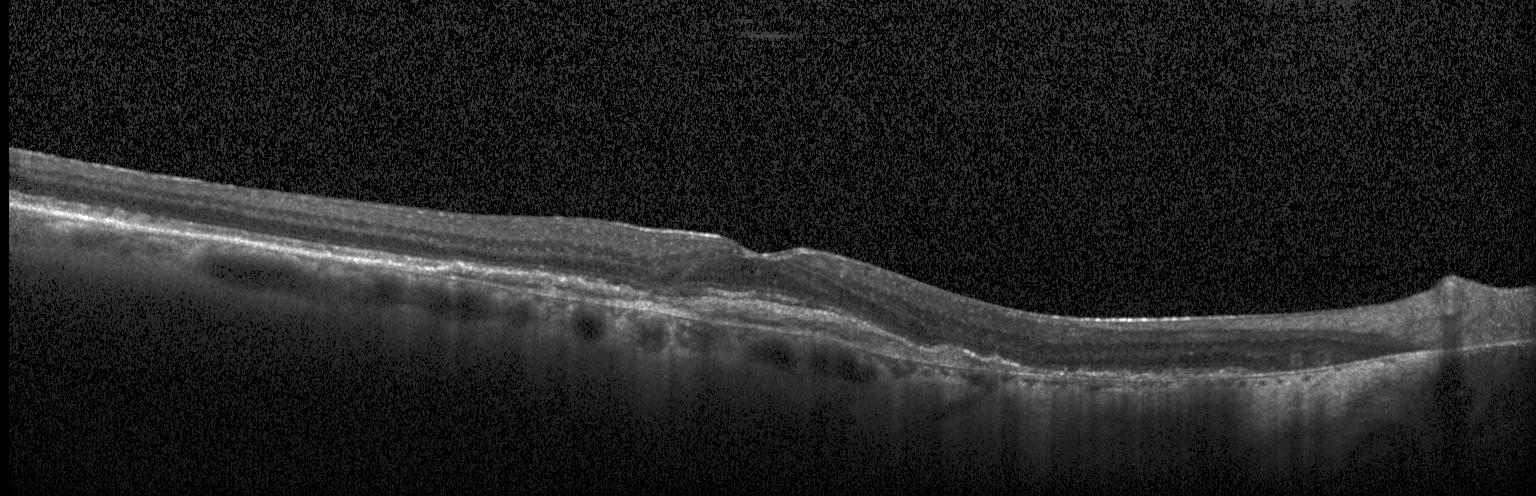 Assessment: a choroidal neovascular membrane.